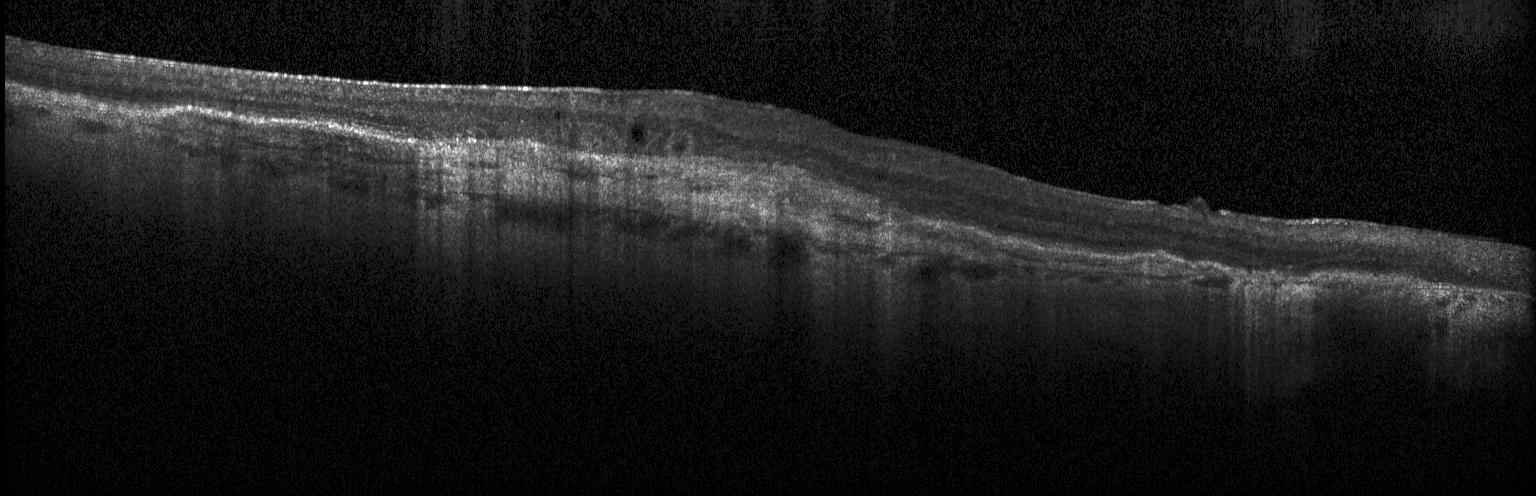

The scan shows a choroidal neovascular membrane.